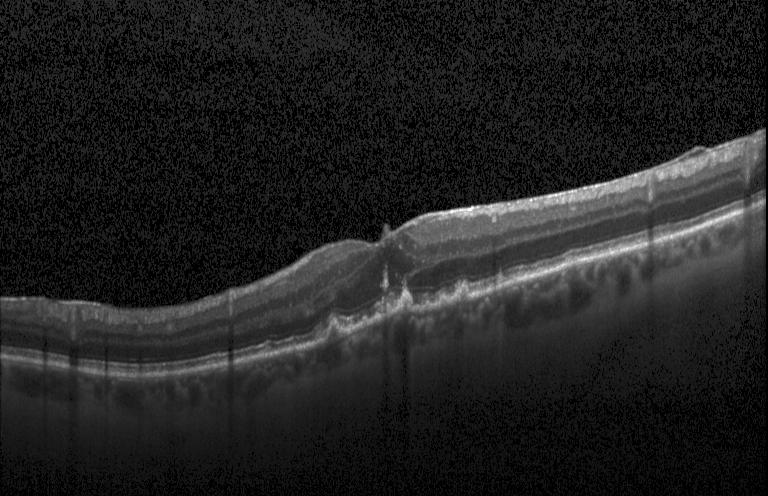

Diagnosis: drusen.